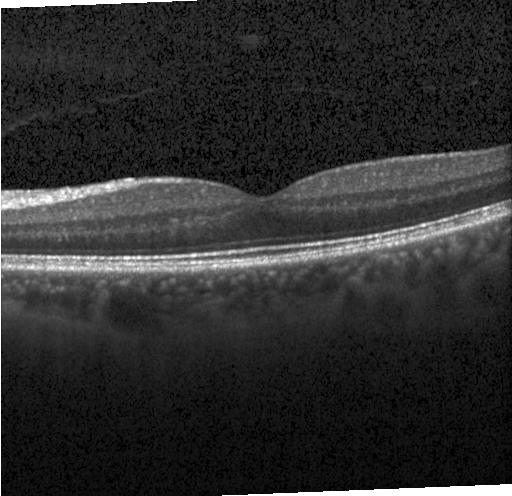 Macular scan. Retinal OCT cross-section — This B-scan demonstrates no evidence of CNV, DME, or drusen.